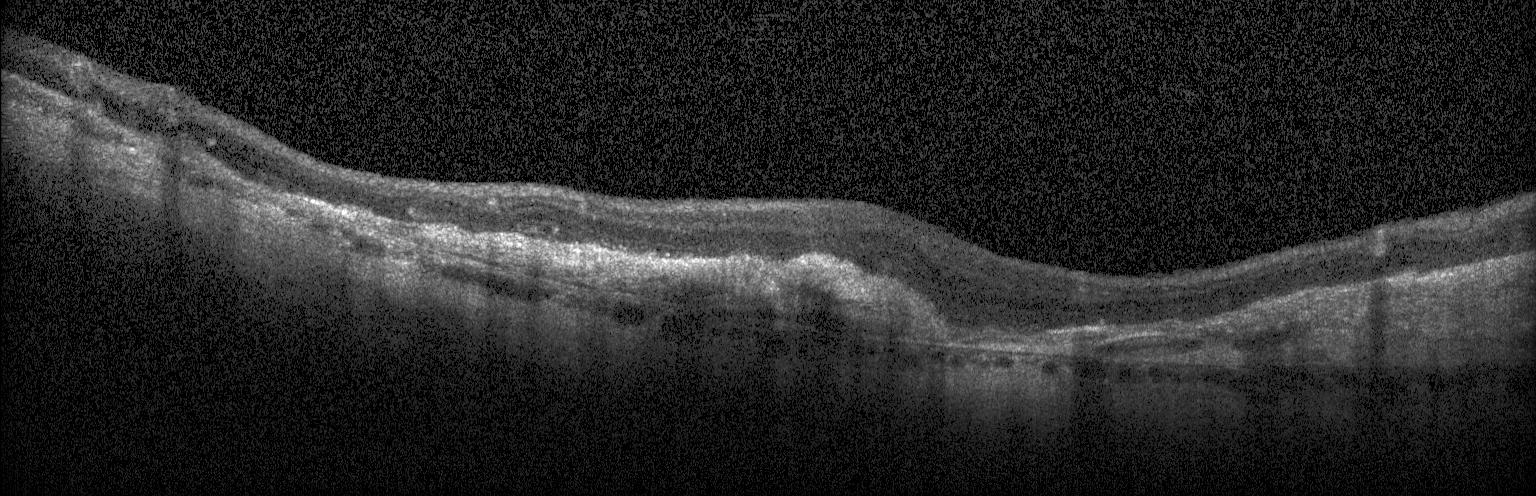 Diagnosis: a choroidal neovascular membrane.